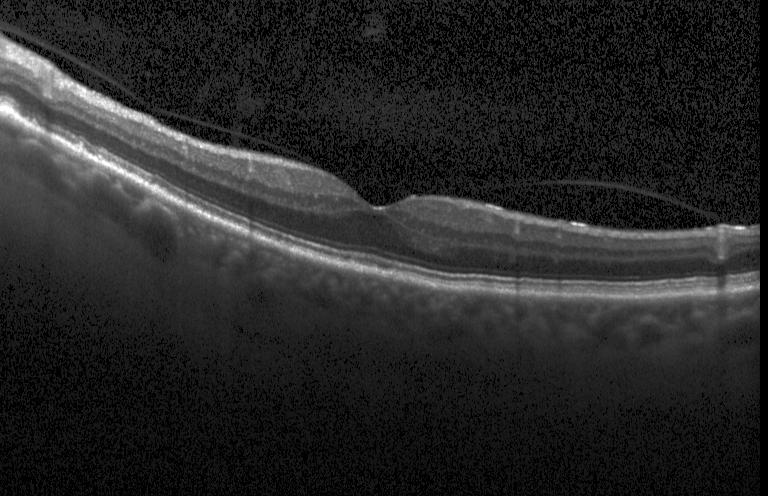

Retinal OCT B-scan · Heidelberg Spectralis OCT system. Diagnosis: no evidence of CNV, DME, or drusen.